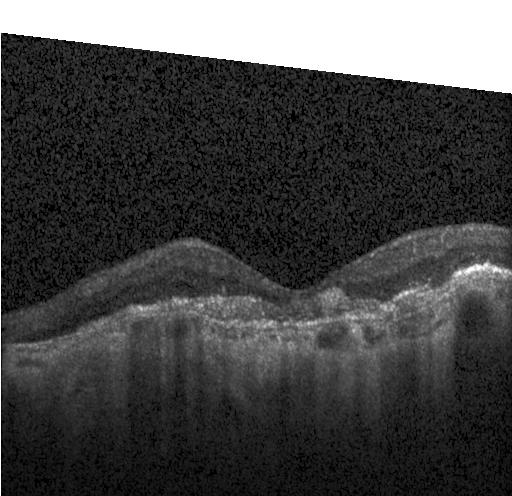

This B-scan demonstrates a choroidal neovascular membrane.